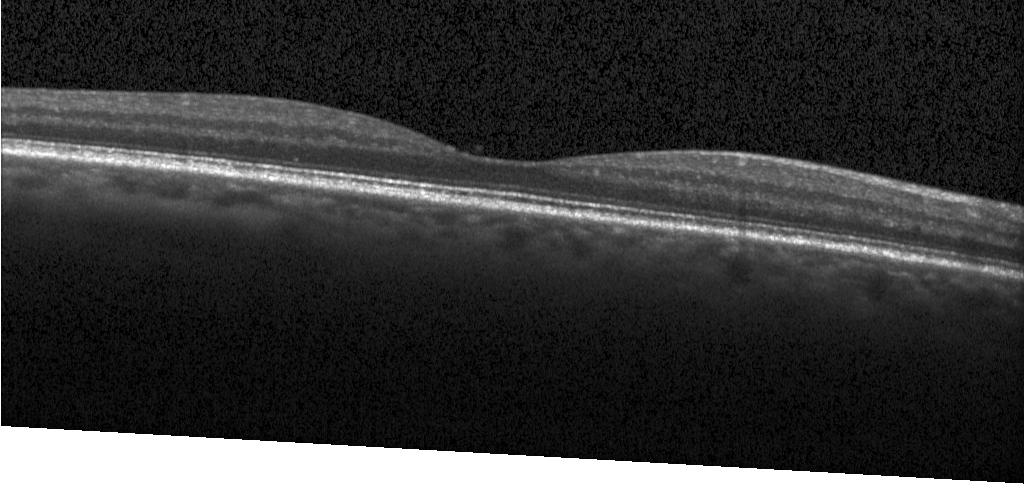

Spectral-domain optical coherence tomography. Through the macula. Heidelberg Spectralis OCT system. Retinal OCT cross-section. Impression: no choroidal neovascularization, no diabetic macular edema, and no drusen.